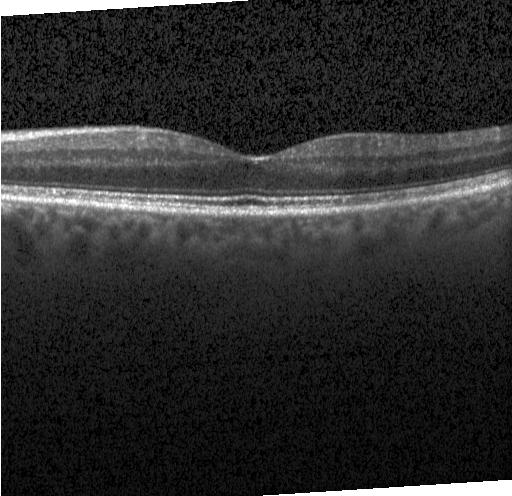
OCT finding: no choroidal neovascularization, no diabetic macular edema, and no drusen.